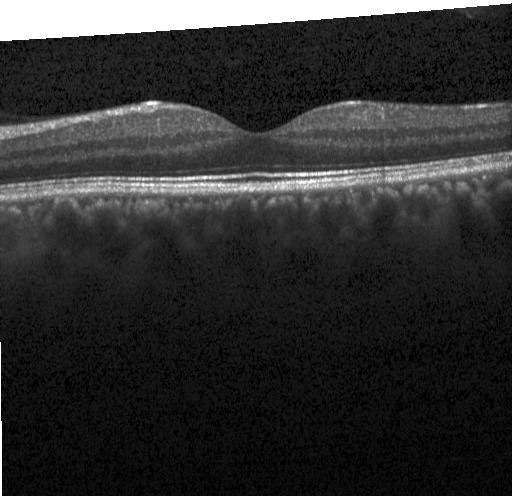
Through the macula; optical coherence tomography B-scan; spectral-domain optical coherence tomography; acquired on a Heidelberg Spectralis. The scan shows neither CNV, DME, nor drusen.